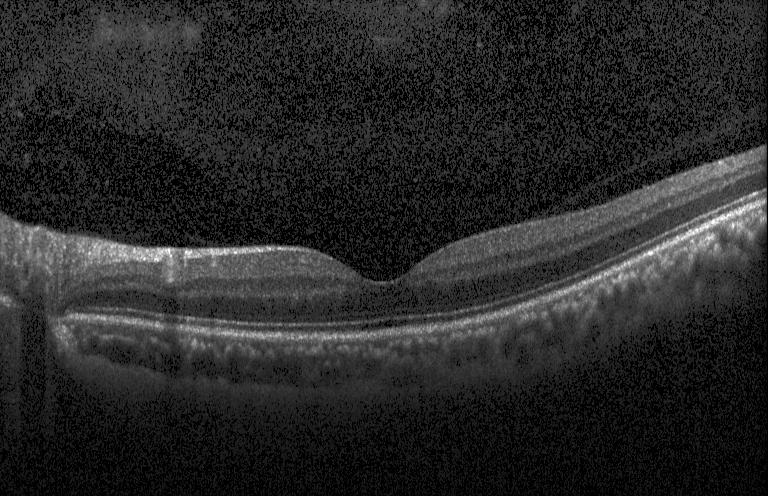

Optical coherence tomography B-scan.
Diagnosis: neither choroidal neovascularization, diabetic macular edema, nor drusen.